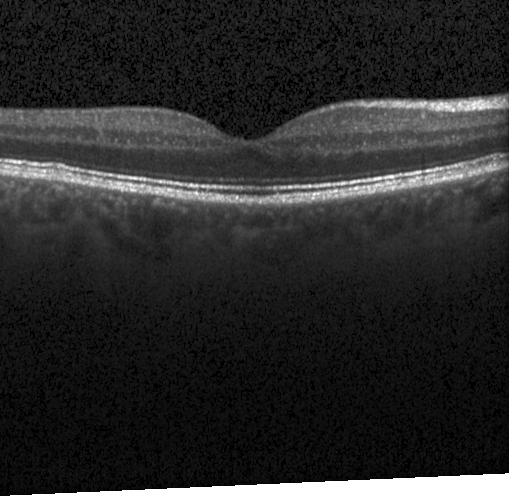 OCT B-scan · centered on the fovea · Heidelberg Spectralis — Finding: neither choroidal neovascularization, diabetic macular edema, nor drusen.